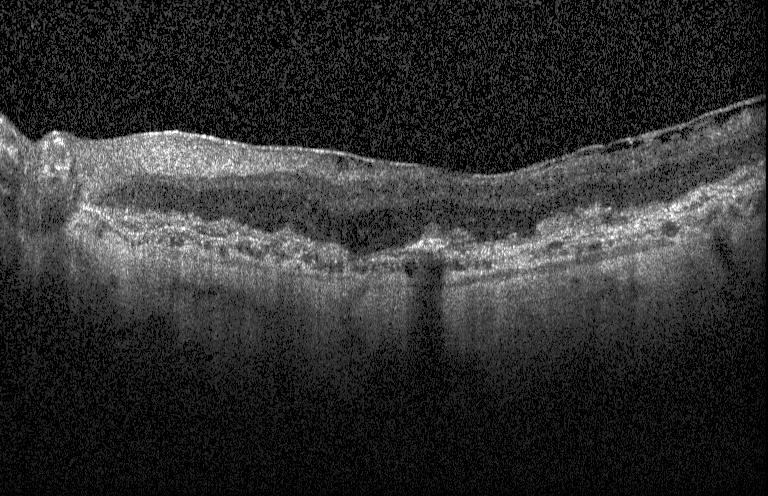

Heidelberg Spectralis OCT system. OCT line scan. Centered on the fovea. Spectral-domain OCT
Impression: CNV.